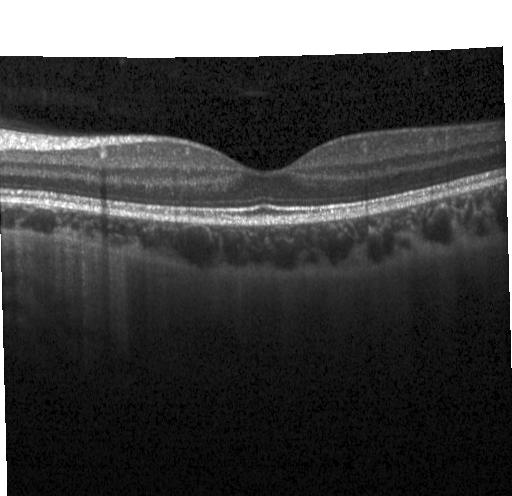

Instrument: Heidelberg Spectralis. OCT B-scan — The scan shows neither choroidal neovascularization, diabetic macular edema, nor drusen.